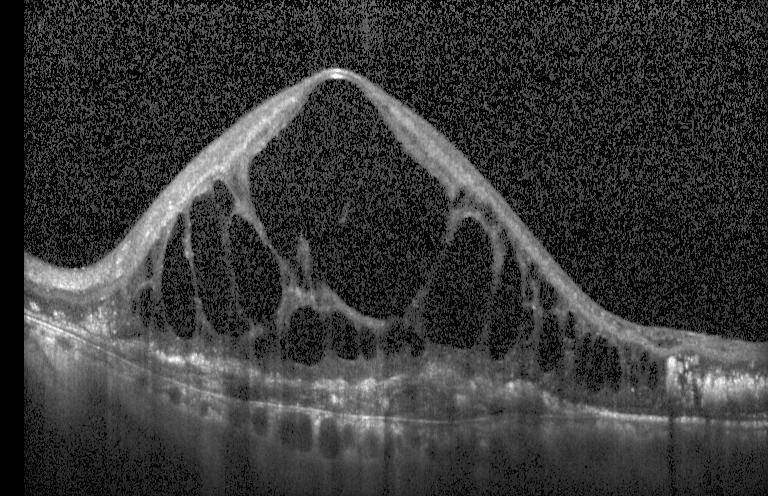 OCT line scan
A choroidal neovascular membrane.